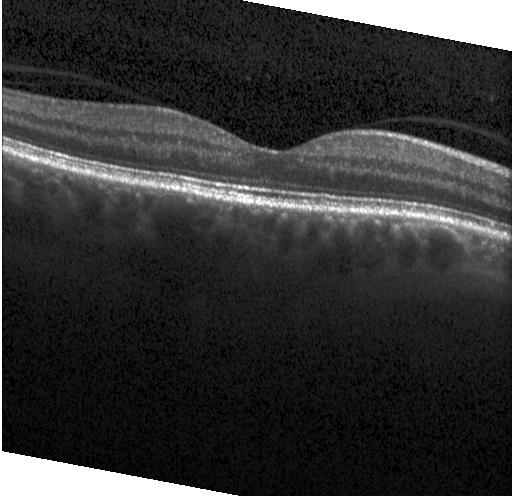

Spectral-domain OCT B-scan: neither choroidal neovascularization, diabetic macular edema, nor drusen.